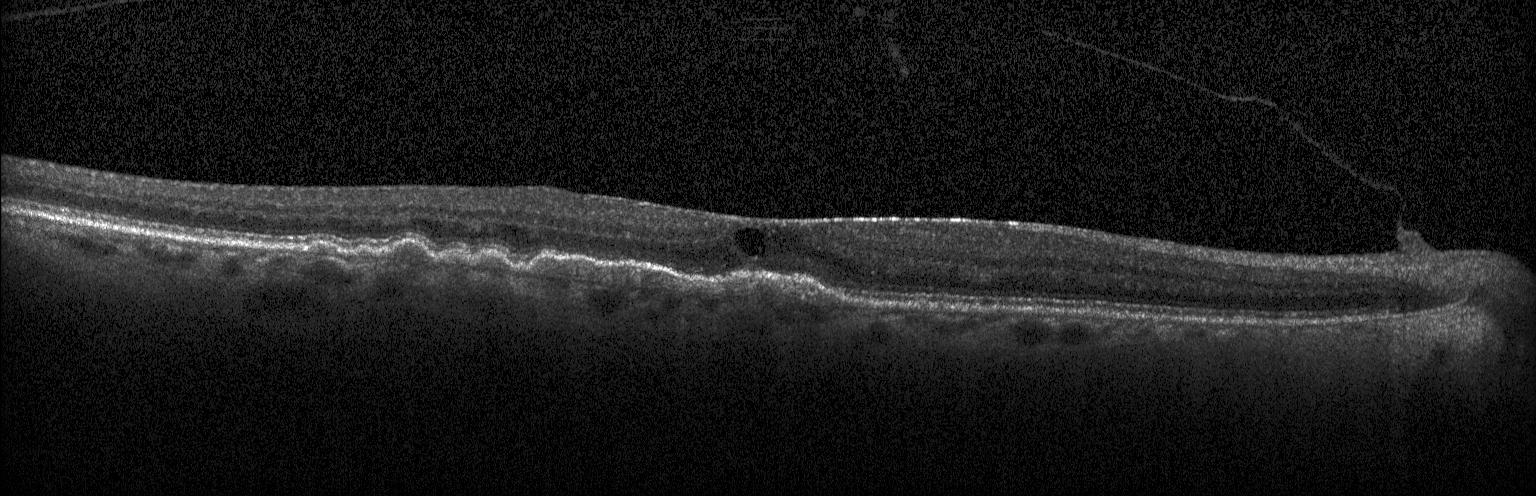
SD-OCT; OCT B-scan; acquired on a Heidelberg Spectralis.
Assessment: CNV.